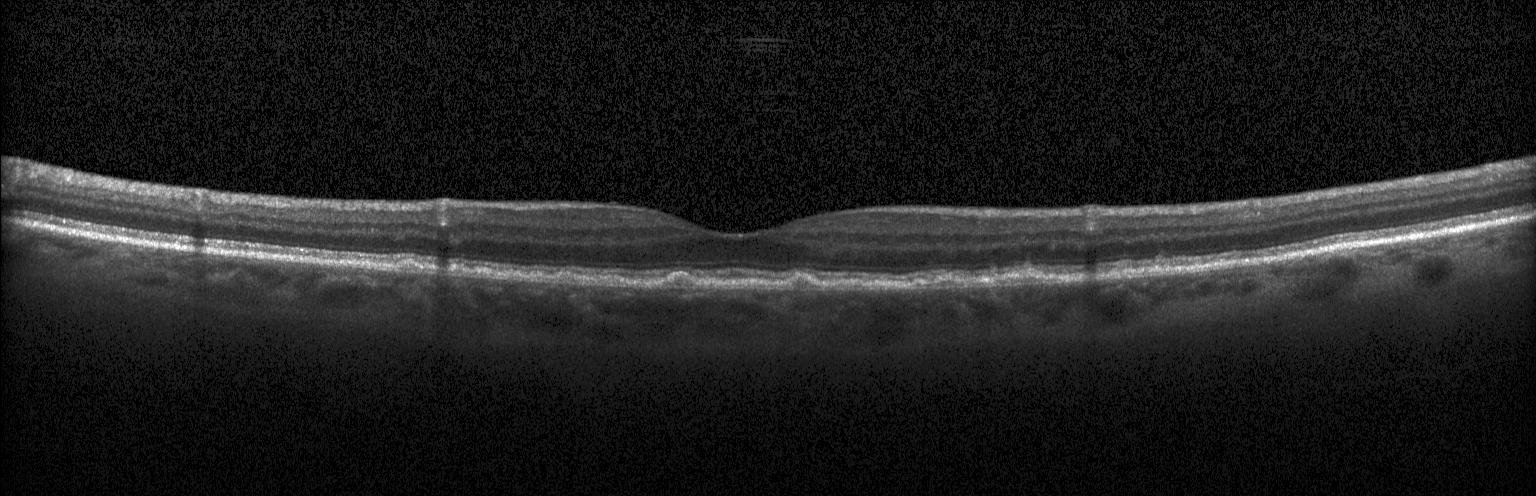
Assessment: sub-RPE drusenoid deposits.